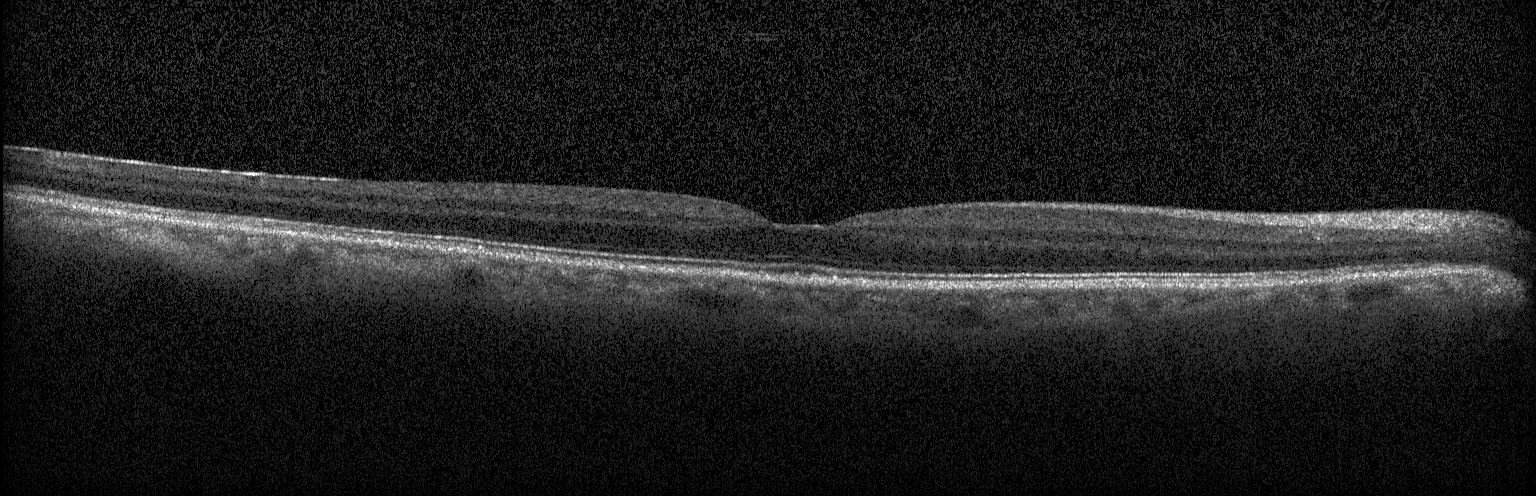 OCT B-scan showing no evidence of CNV, DME, or drusen.